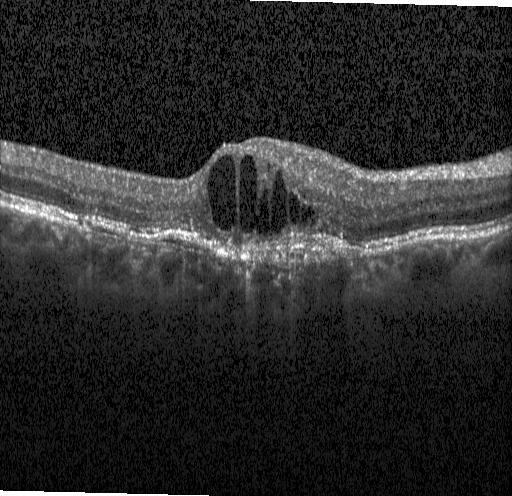
OCT B-scan showing a choroidal neovascular membrane.